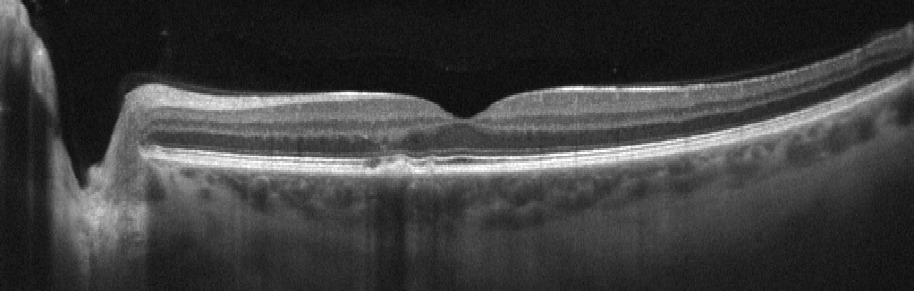

Oculus dexter · optical coherence tomography scan. Dx: AMD.